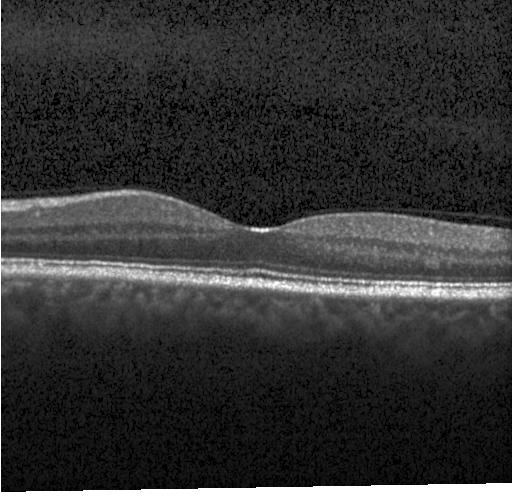
SD-OCT · optical coherence tomography B-scan.
The scan shows no CNV, DME, or drusen.